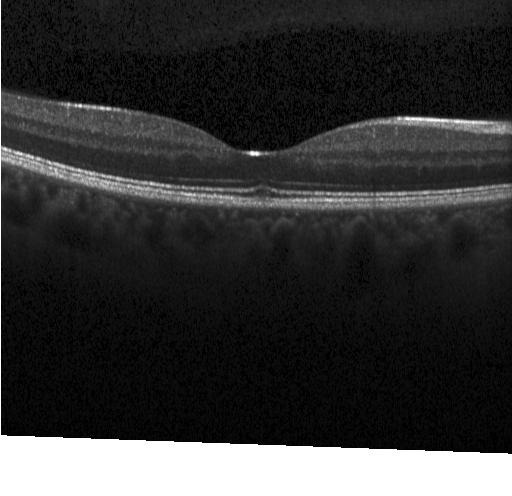

Optical coherence tomography B-scan — The scan shows neither choroidal neovascularization, diabetic macular edema, nor drusen.